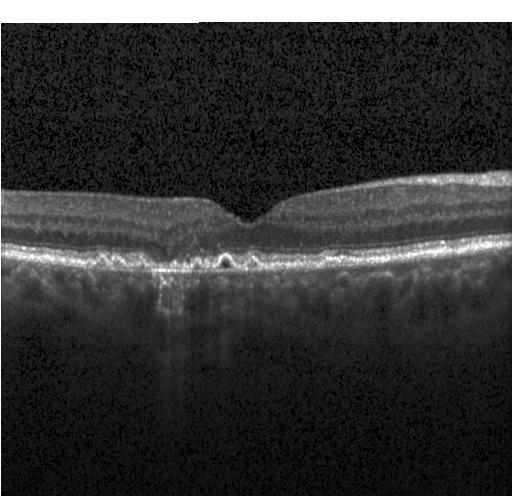
Macular OCT: a choroidal neovascular membrane.